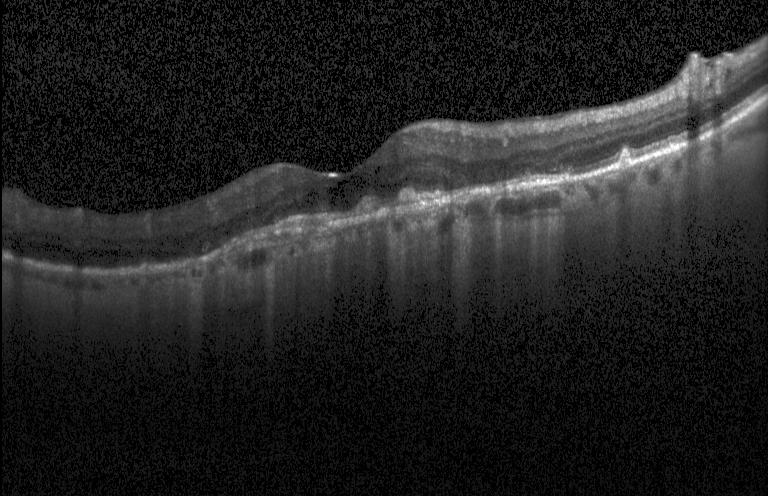

This B-scan demonstrates CNV.